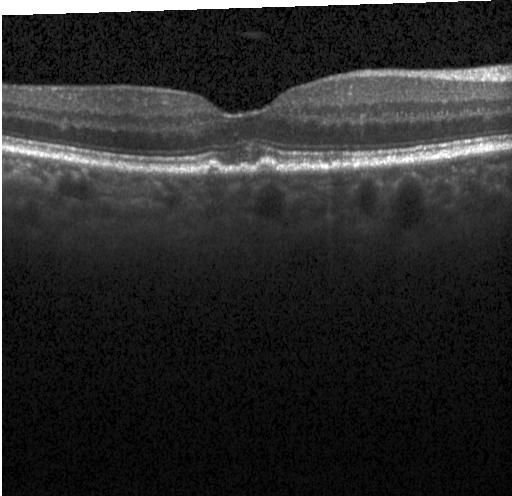

OCT line scan.
Assessment: multiple drusen.